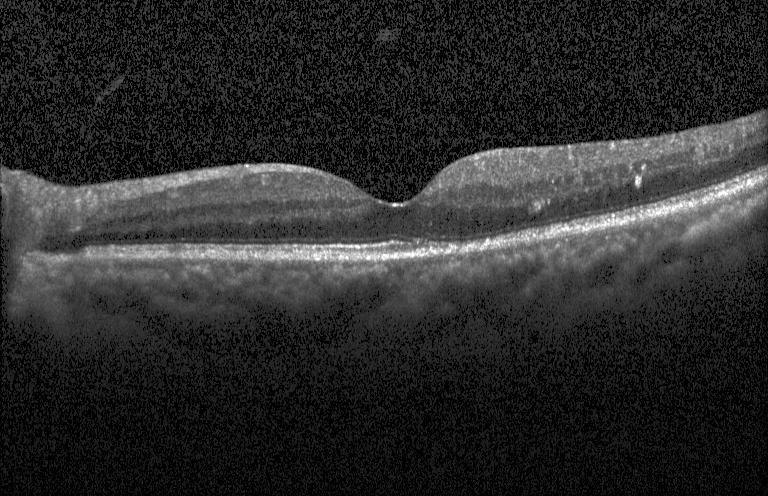
Spectral-domain OCT B-scan: DME.